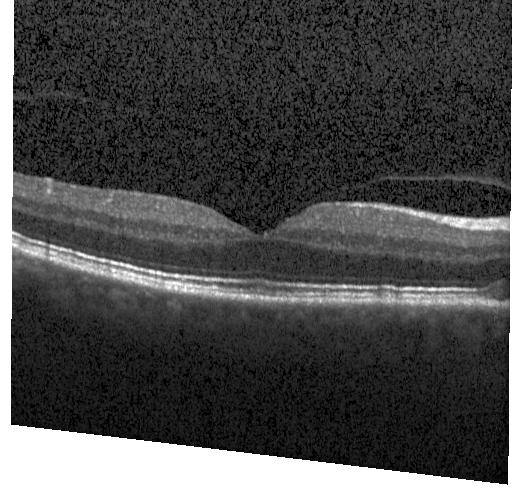
Finding: no choroidal neovascularization, diabetic macular edema, or drusen.